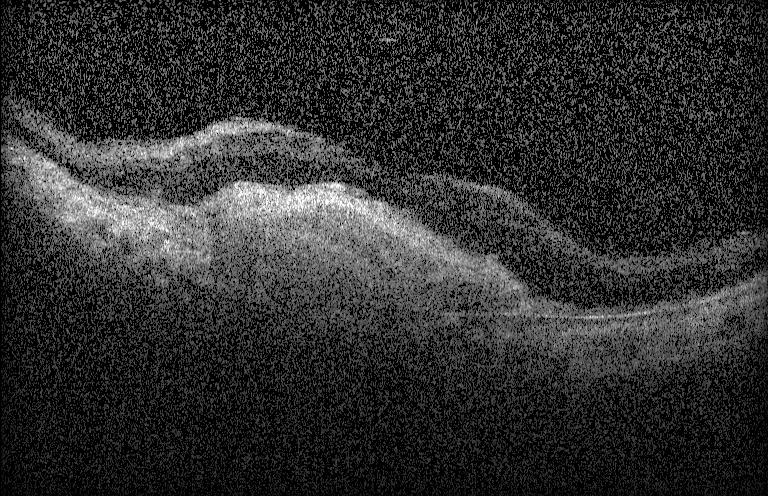

Retinal OCT cross-section; SD-OCT — OCT finding: a choroidal neovascular membrane.